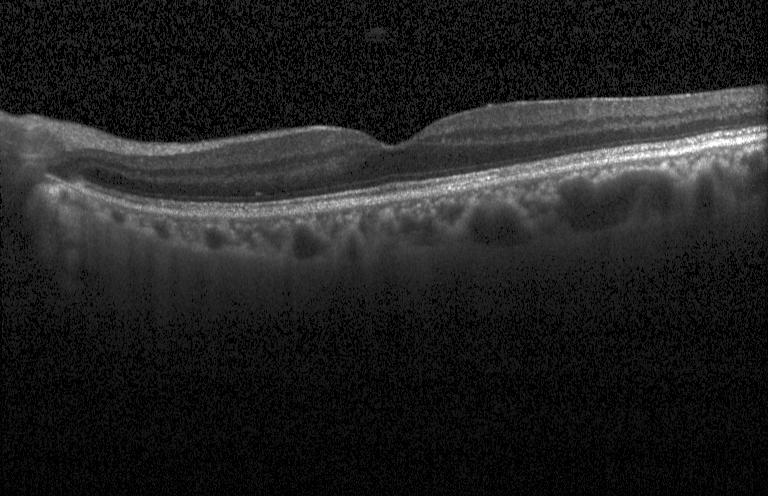
OCT B-scan; SD-OCT; centered on the fovea — Impression: no evidence of CNV, DME, or drusen.